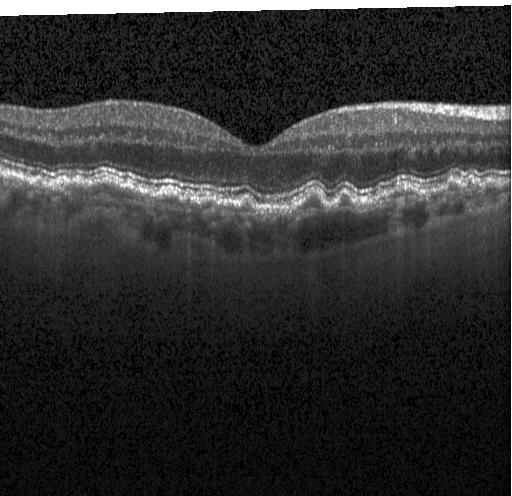

Dx: multiple drusen.